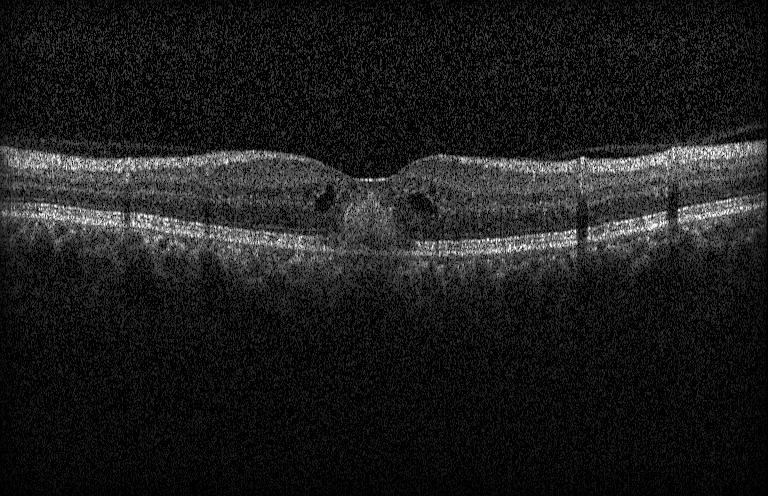
Retinal OCT cross-section showing a choroidal neovascular membrane.